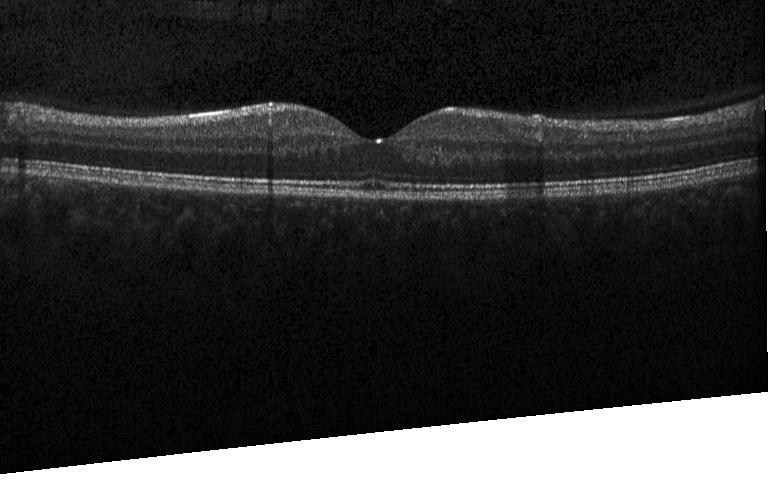
Retinal OCT B-scan · spectral-domain OCT · Heidelberg Spectralis · through the macula — Diagnosis: no evidence of choroidal neovascularization, diabetic macular edema, or drusen.